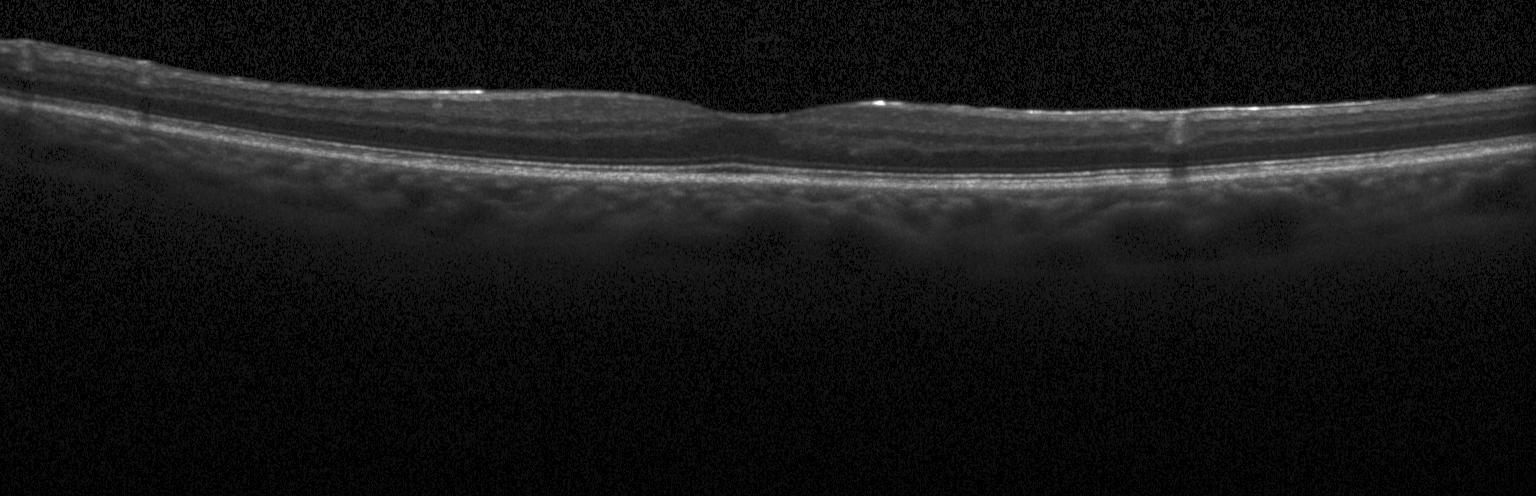

Impression: neither choroidal neovascularization, diabetic macular edema, nor drusen.